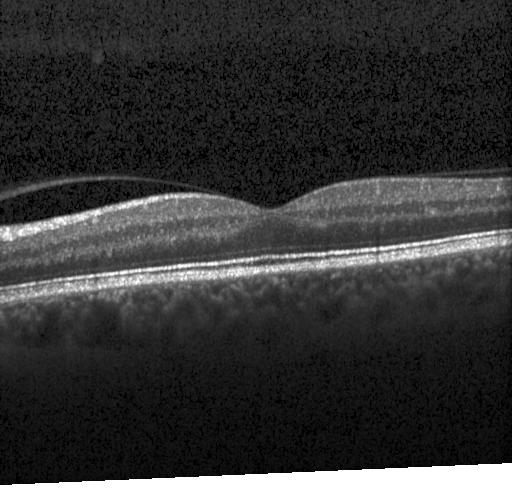

Through the macula · retinal OCT cross-section · spectral-domain OCT · Heidelberg Spectralis.
Finding: no choroidal neovascularization, no diabetic macular edema, and no drusen.